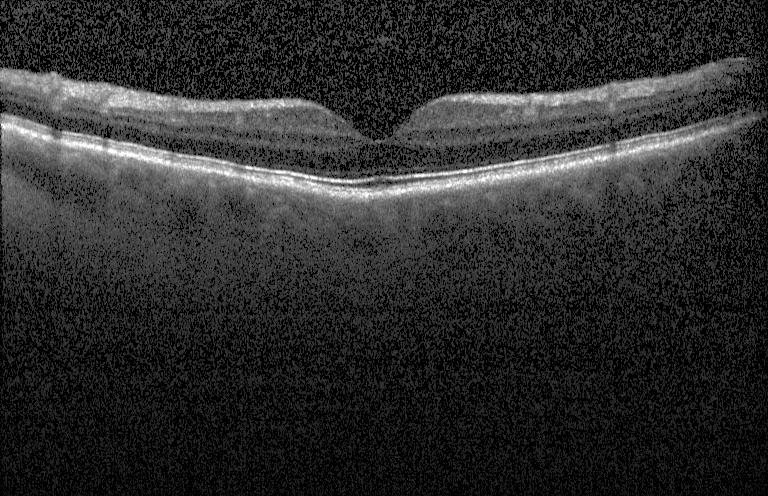

Heidelberg Spectralis · OCT B-scan · SD-OCT · macular scan — The scan shows no evidence of choroidal neovascularization, diabetic macular edema, or drusen.